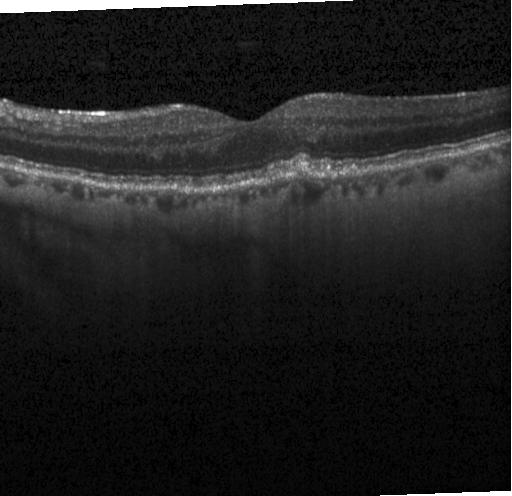
Macular OCT demonstrating drusen.